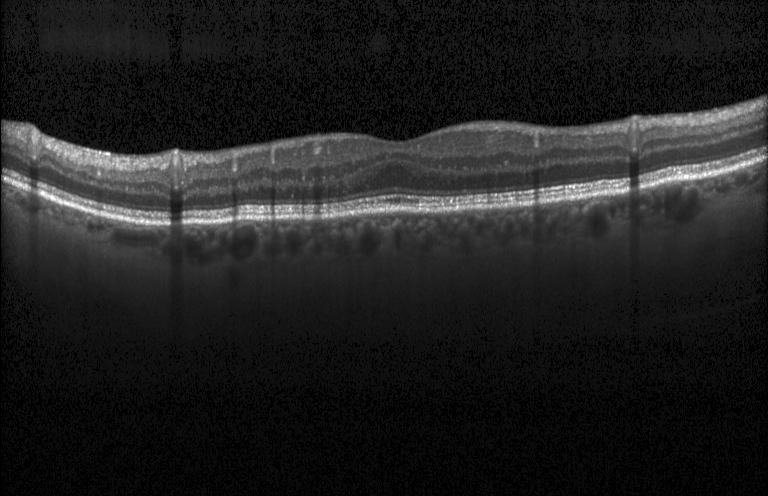
SD-OCT; retinal OCT B-scan; macular scan.
Diagnosis: no choroidal neovascularization, no diabetic macular edema, and no drusen.